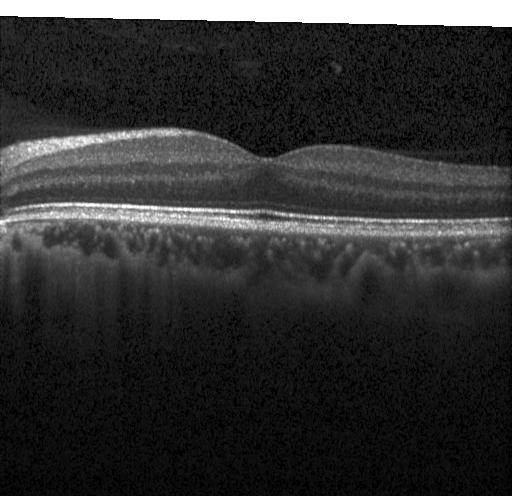

Retinal OCT B-scan; Heidelberg Spectralis — OCT finding: no choroidal neovascularization, no diabetic macular edema, and no drusen.